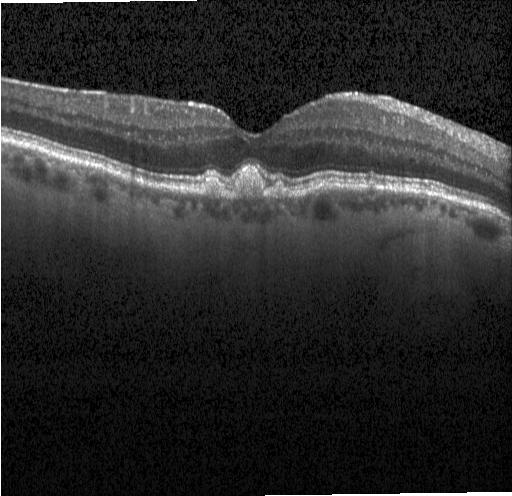 Sub-RPE drusenoid deposits.